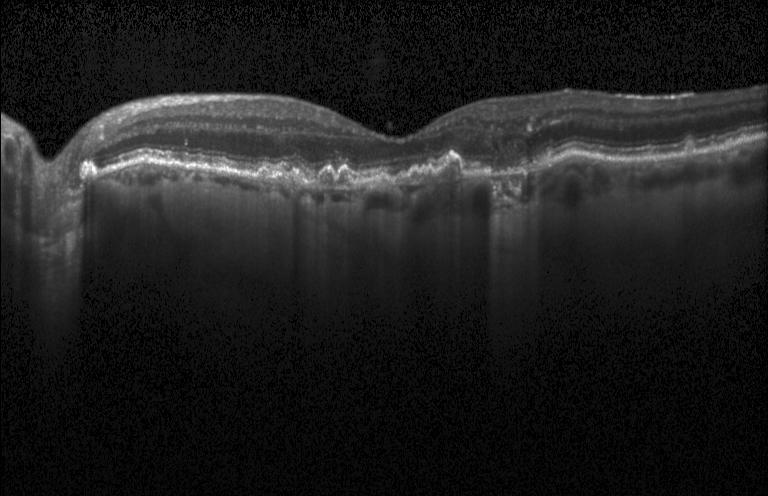

Retinal OCT cross-section; through the macula; Heidelberg Spectralis OCT system; SD-OCT.
A choroidal neovascular membrane.